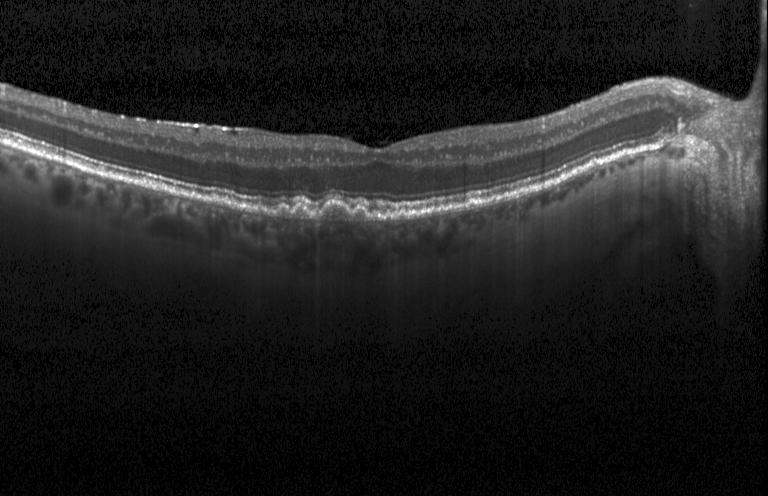 Spectral-domain OCT B-scan: sub-RPE drusenoid deposits.